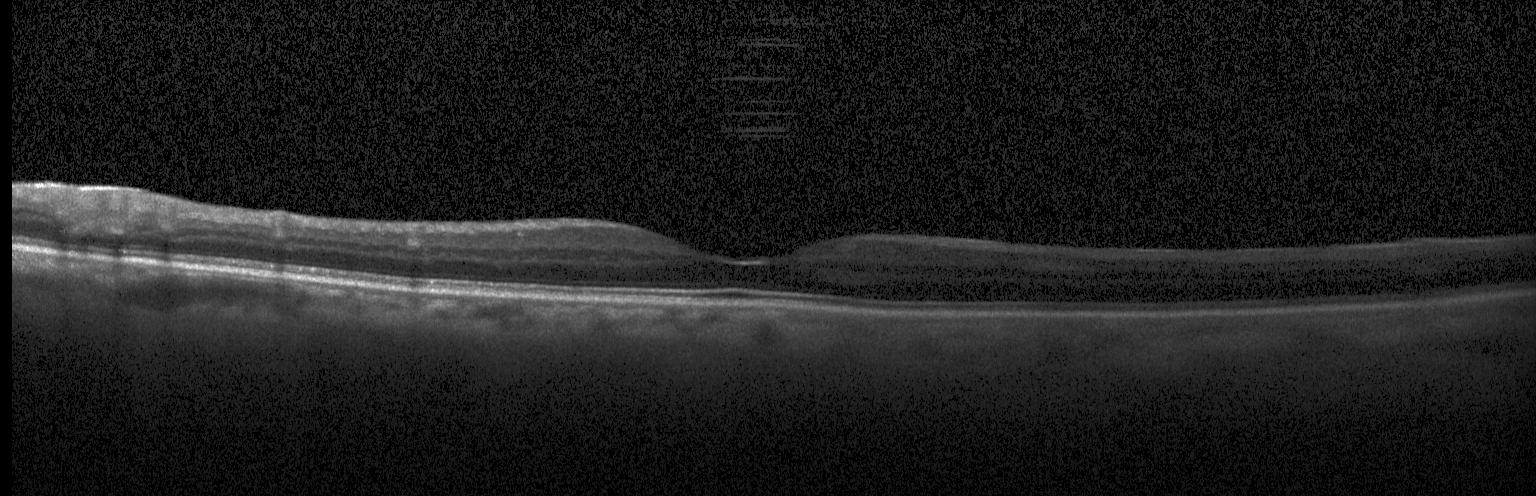 Retinal OCT cross-section, Heidelberg Spectralis. Impression: no CNV, DME, or drusen.